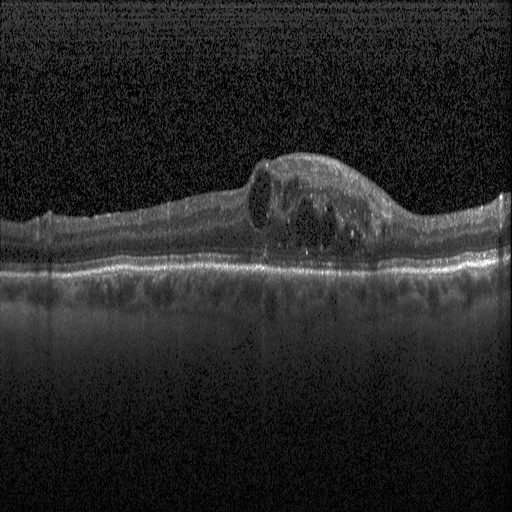 OCT line scan.
DME.